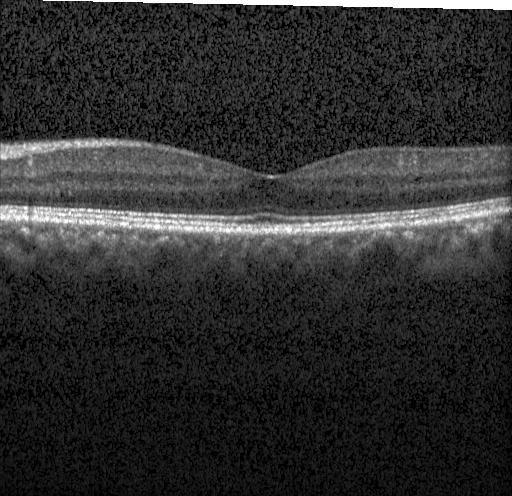
Spectral-domain optical coherence tomography; optical coherence tomography scan — The scan shows no choroidal neovascularization, no diabetic macular edema, and no drusen.